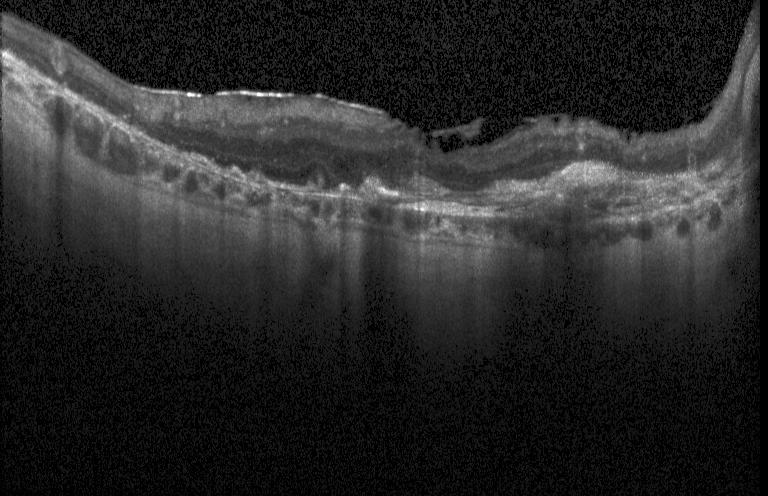

Finding: choroidal neovascularization (CNV).